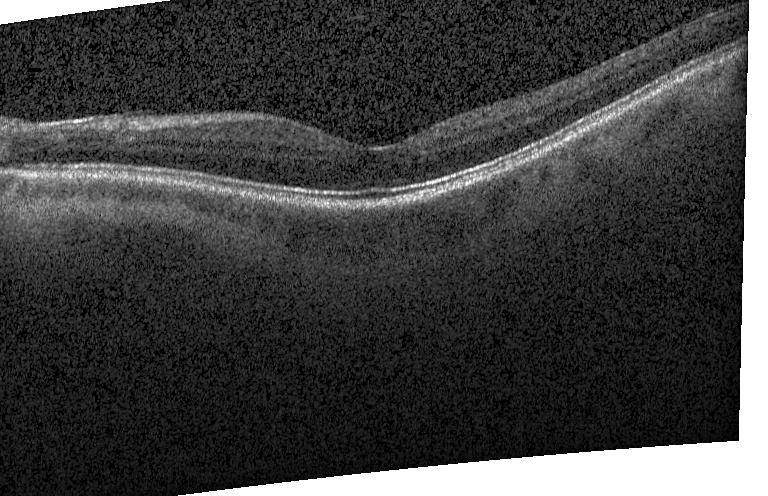

Heidelberg Spectralis OCT system · optical coherence tomography B-scan.
Diagnosis: no choroidal neovascularization, diabetic macular edema, or drusen.